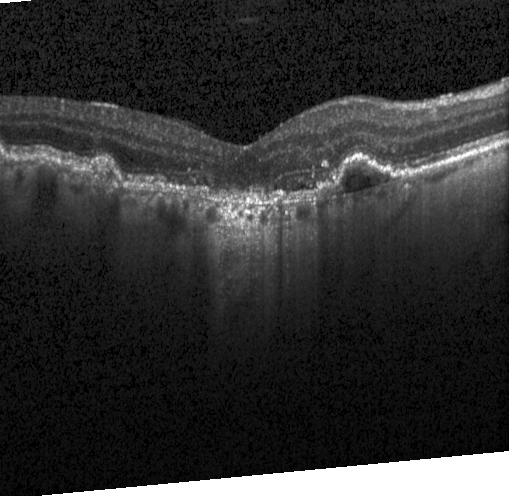

Optical coherence tomography scan — The scan shows CNV.